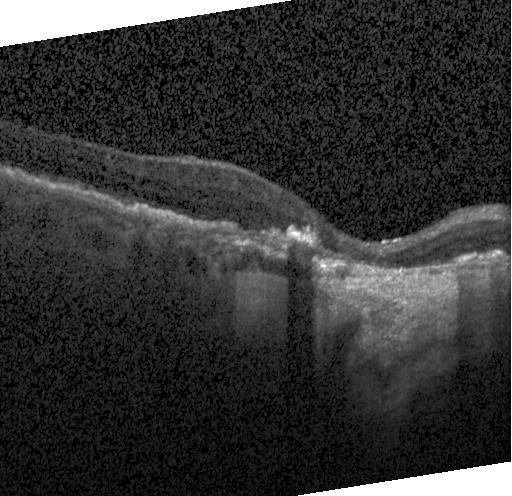
OCT line scan. Spectral-domain OCT. Heidelberg Spectralis. Through the macula.
Impression: choroidal neovascularization.